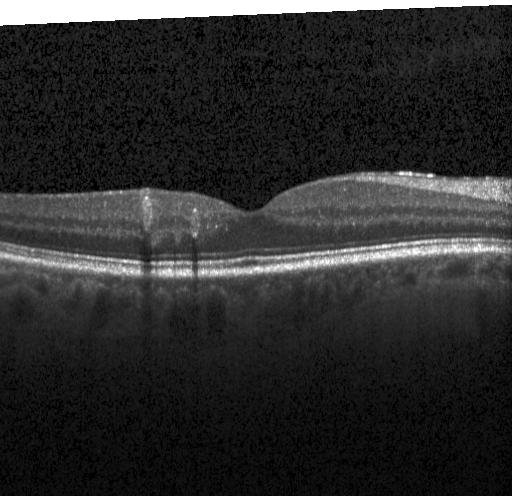 Impression: no CNV, no DME, and no drusen.